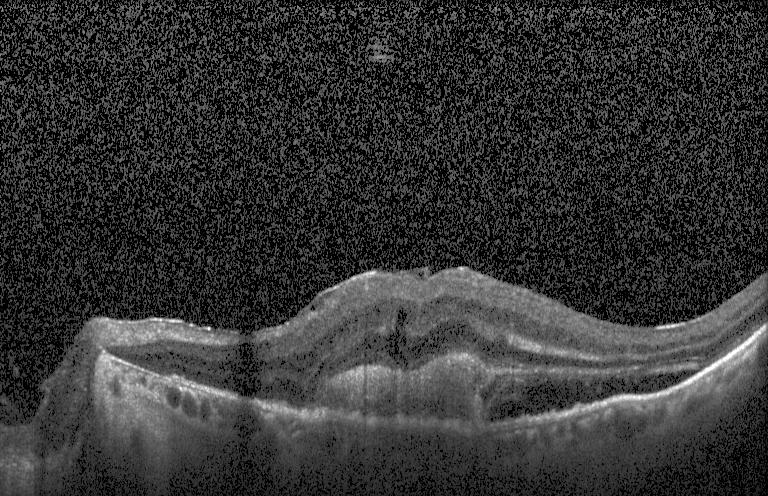

SD-OCT; optical coherence tomography scan. Diagnosis: a choroidal neovascular membrane.